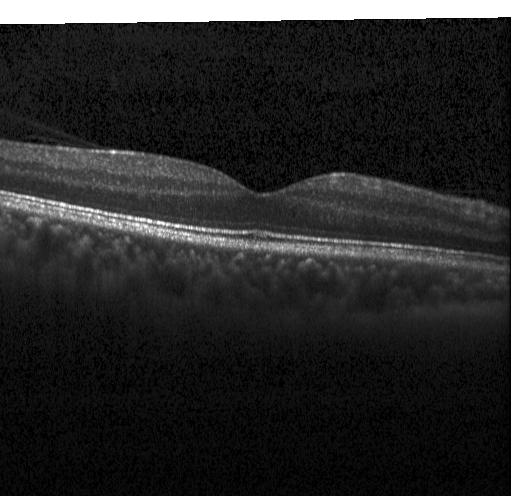 OCT finding: no CNV, DME, or drusen.